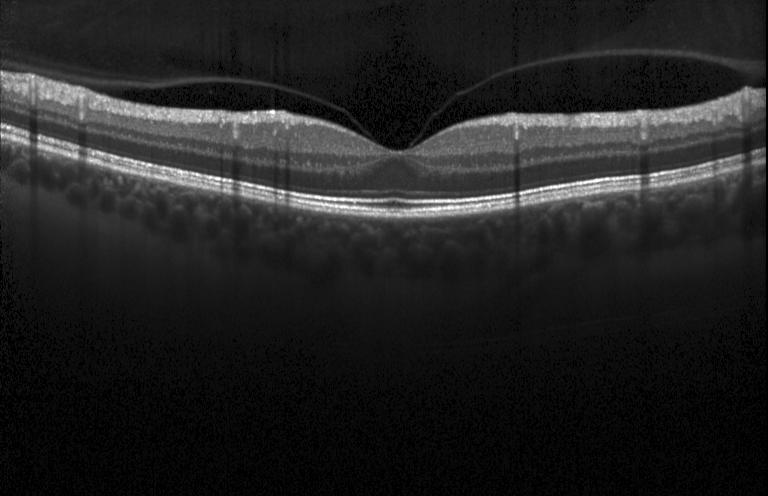
Macular OCT: no choroidal neovascularization, no diabetic macular edema, and no drusen.